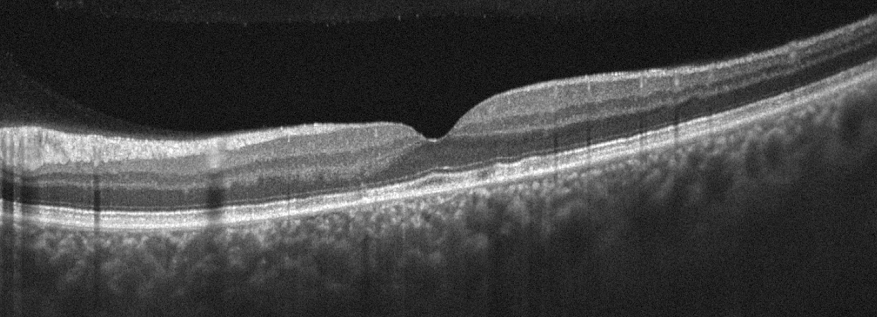

OCT B-scan
Assessment: age-related macular degeneration.